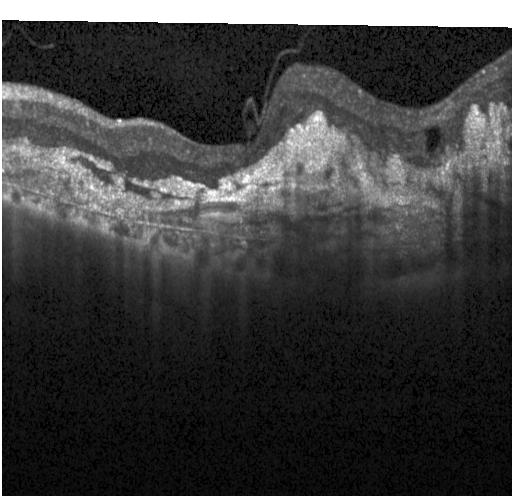

Diagnosis: choroidal neovascularization.